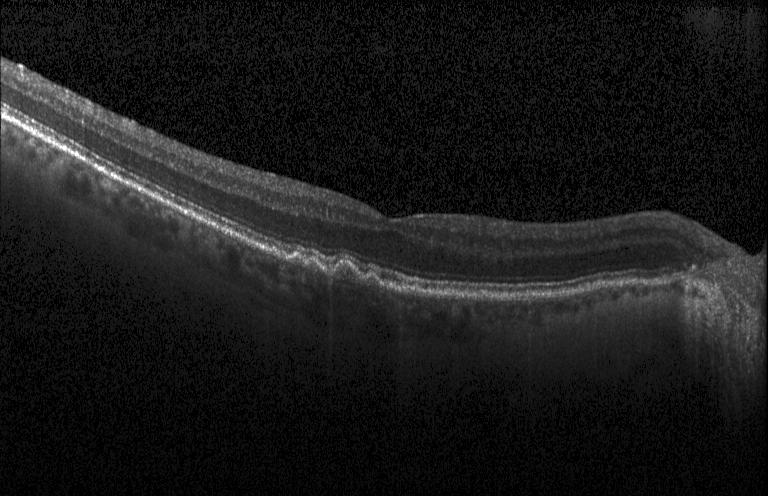
Multiple drusen.